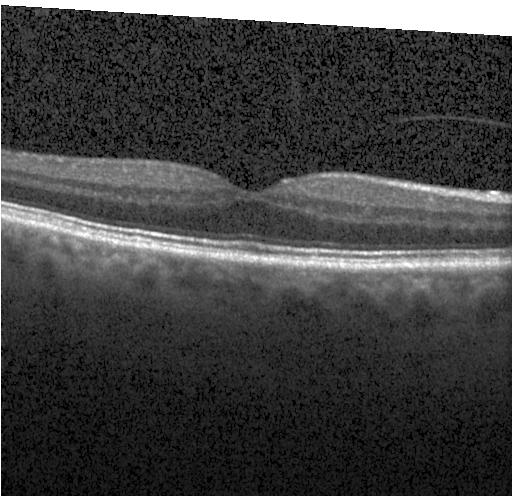
Diagnosis: no evidence of CNV, DME, or drusen.